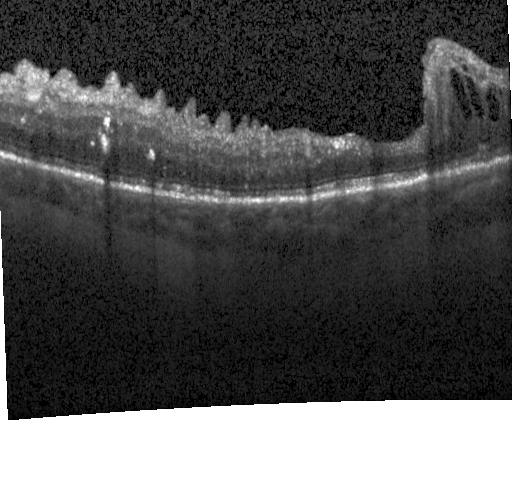

Acquired on a Heidelberg Spectralis; OCT B-scan.
The scan shows DME.